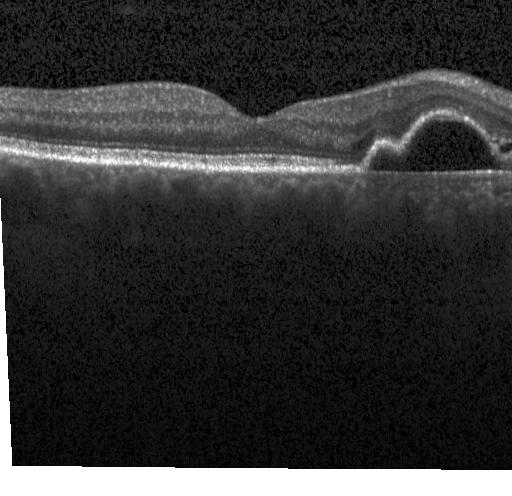

Acquired on a Heidelberg Spectralis. Spectral-domain OCT. OCT B-scan.
This B-scan demonstrates choroidal neovascularization.